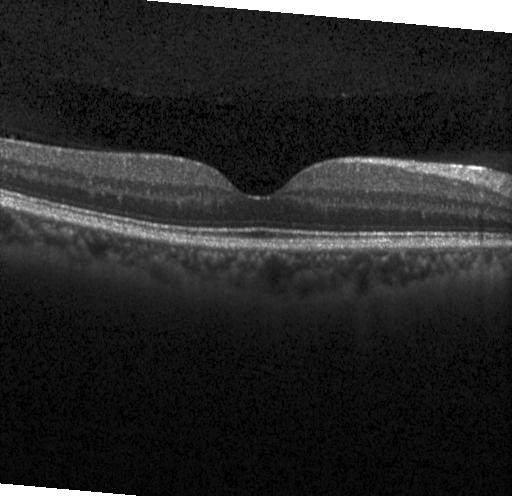 Finding: no choroidal neovascularization, no diabetic macular edema, and no drusen.